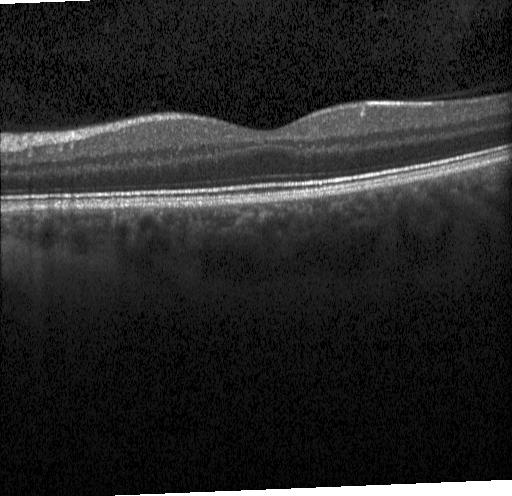 Spectral-domain OCT; optical coherence tomography scan; Heidelberg Spectralis
Finding: no CNV, no DME, and no drusen.